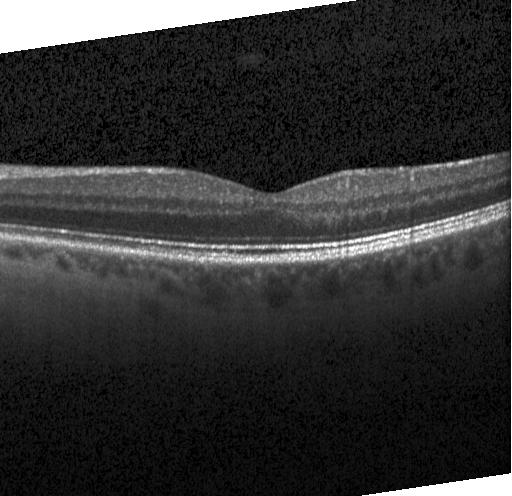 Horizontal scan through the fovea. Retinal OCT B-scan — Impression: no evidence of CNV, DME, or drusen.